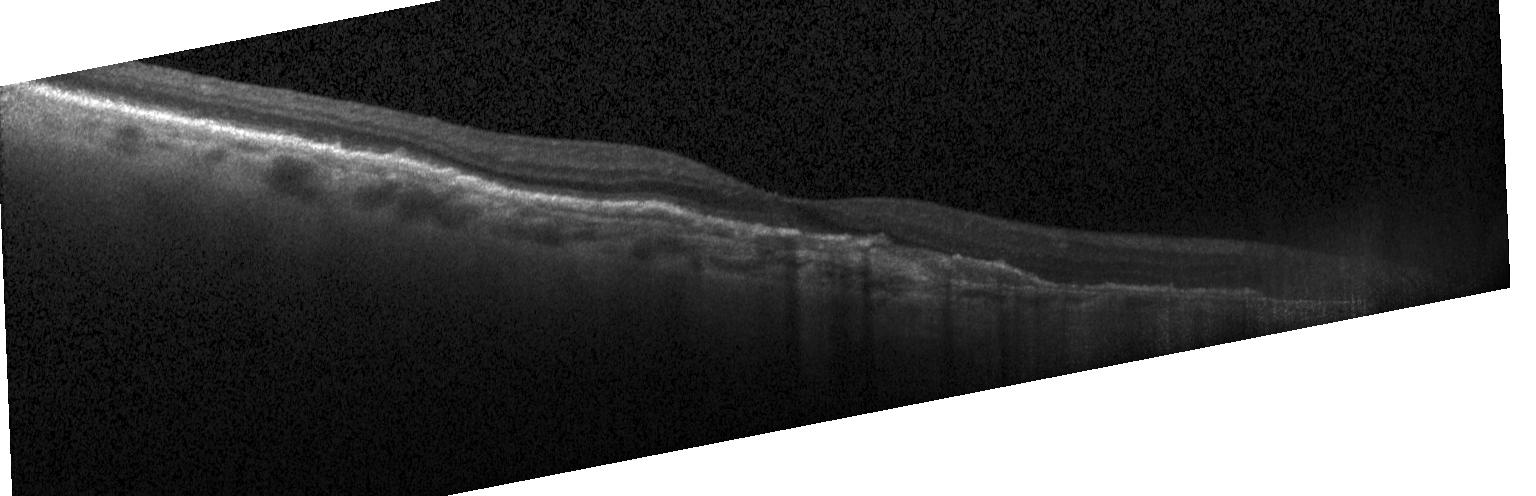 SD-OCT. Instrument: Heidelberg Spectralis. Retinal OCT B-scan. Fovea-centered
Dx: choroidal neovascularization.